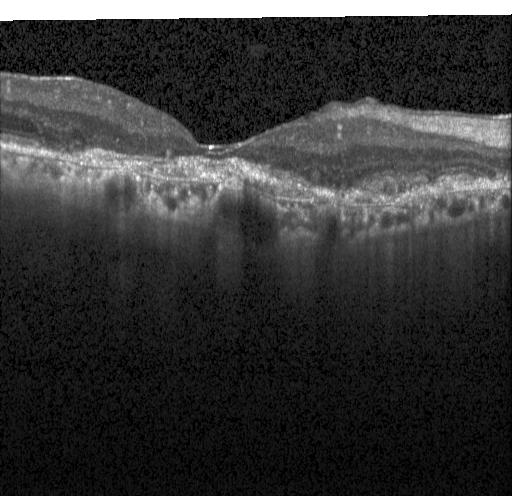 Finding: a choroidal neovascular membrane.